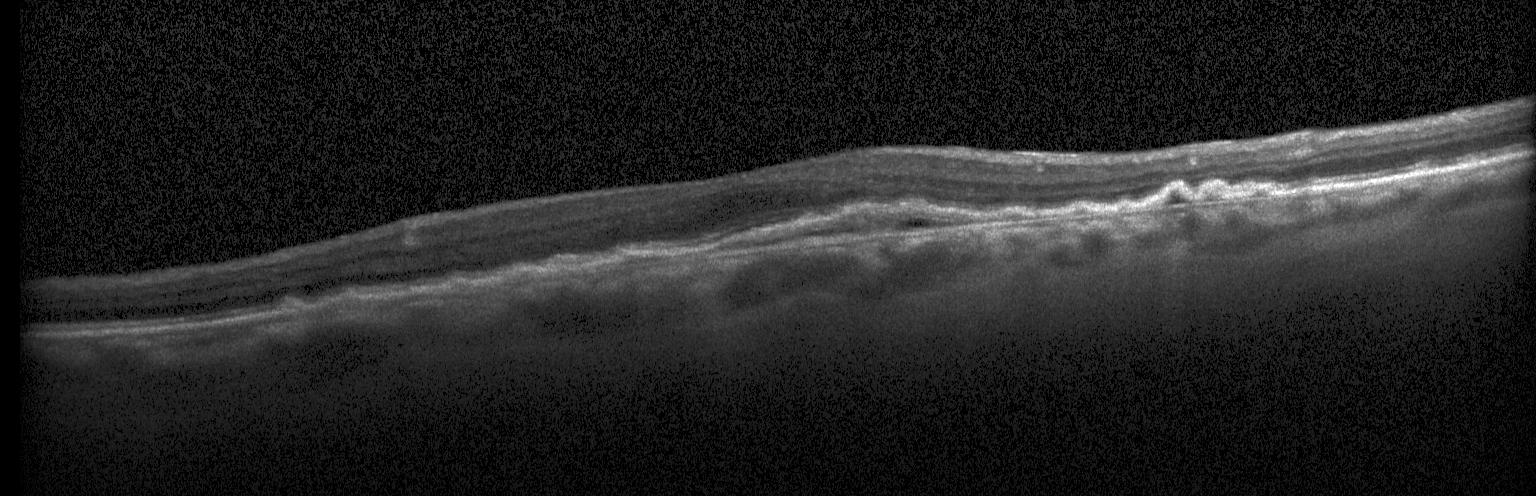
SD-OCT; retinal OCT B-scan; Heidelberg Spectralis
Impression: a choroidal neovascular membrane.